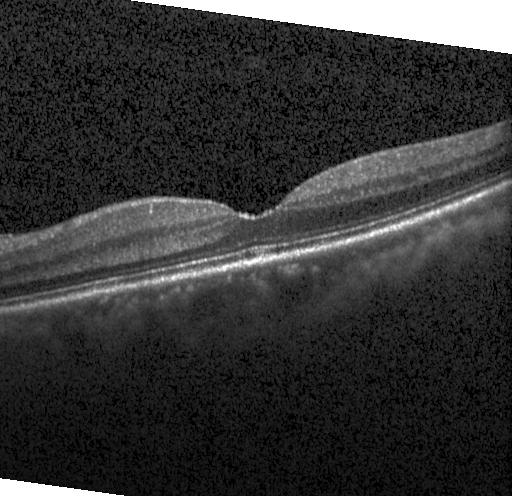 Diagnosis: no choroidal neovascularization, diabetic macular edema, or drusen.